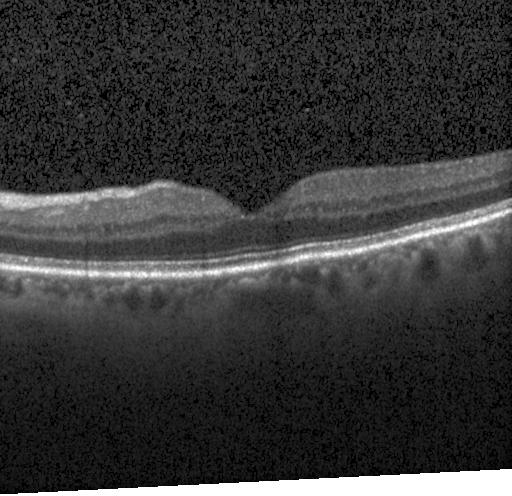
Macular OCT: no CNV, DME, or drusen.